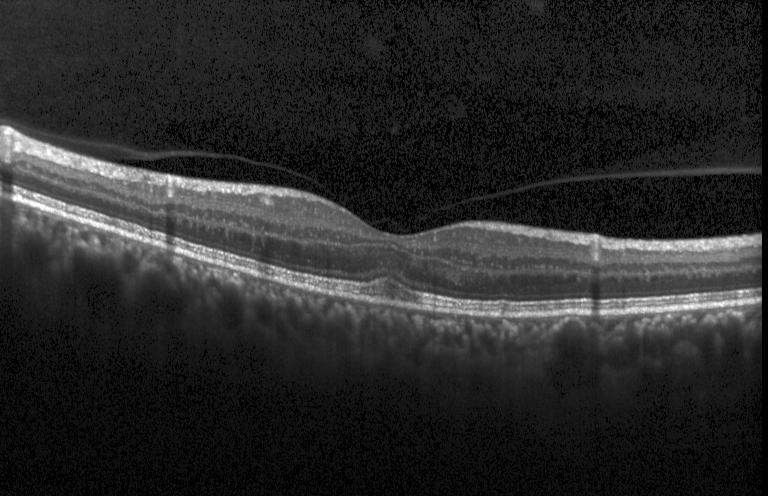 Heidelberg Spectralis. Macular scan. Retinal OCT cross-section. SD-OCT.
This B-scan demonstrates a choroidal neovascular membrane.